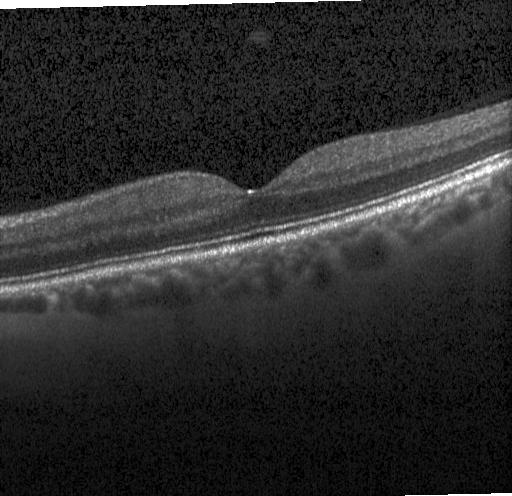
Retinal OCT cross-section. Diagnosis: no choroidal neovascularization, no diabetic macular edema, and no drusen.